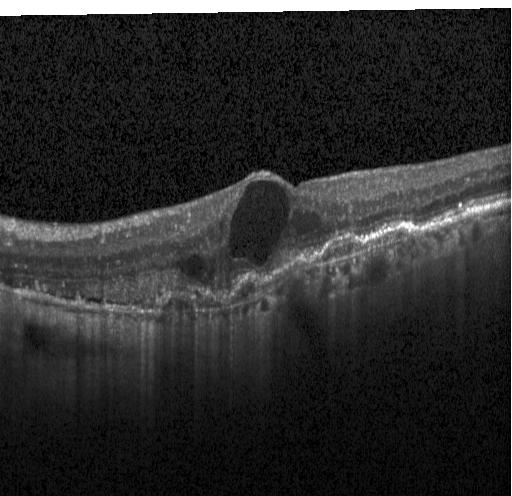

Heidelberg Spectralis; spectral-domain optical coherence tomography; retinal OCT B-scan.
Diagnosis: choroidal neovascularization (CNV).